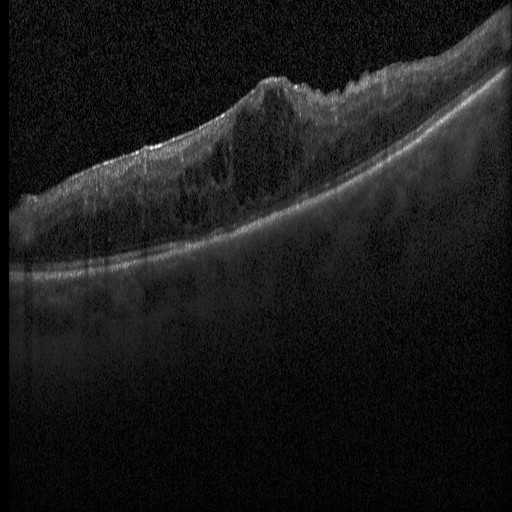 Spectral-domain optical coherence tomography; acquired on a Heidelberg Spectralis; OCT B-scan. Diagnosis: DME.